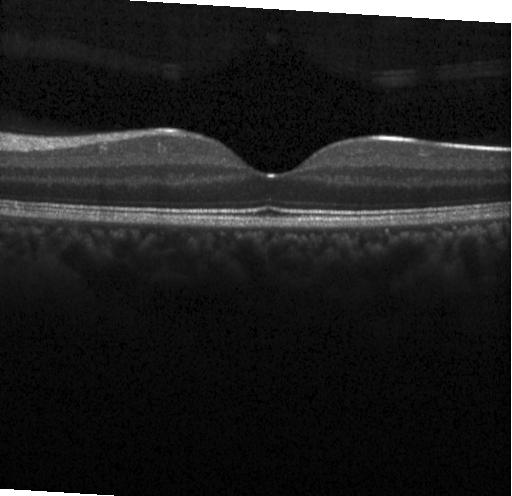

Instrument: Heidelberg Spectralis, SD-OCT, OCT B-scan, macular scan. Macular OCT: neither choroidal neovascularization, diabetic macular edema, nor drusen.